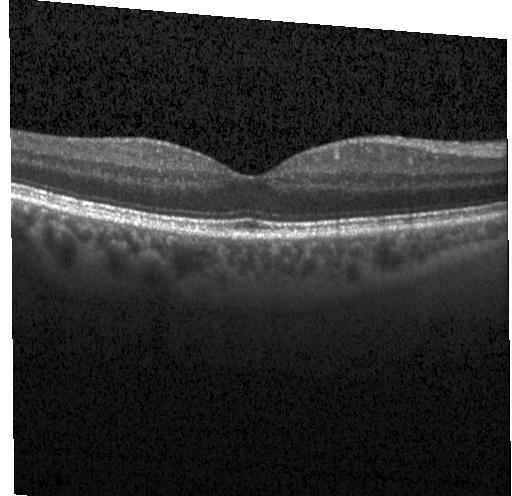
OCT B-scan, instrument: Heidelberg Spectralis. Impression: no CNV, DME, or drusen.